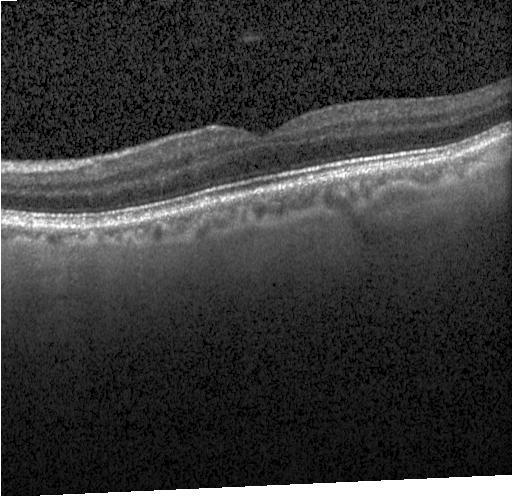

Macular OCT demonstrating neither choroidal neovascularization, diabetic macular edema, nor drusen.